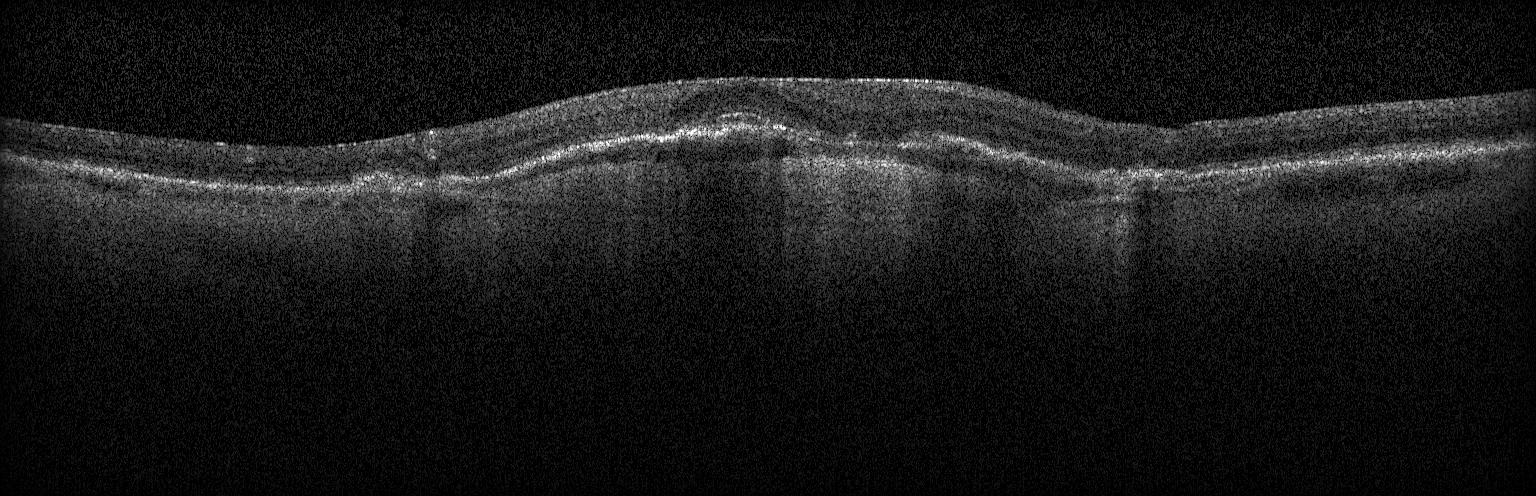

Macular OCT: a choroidal neovascular membrane.